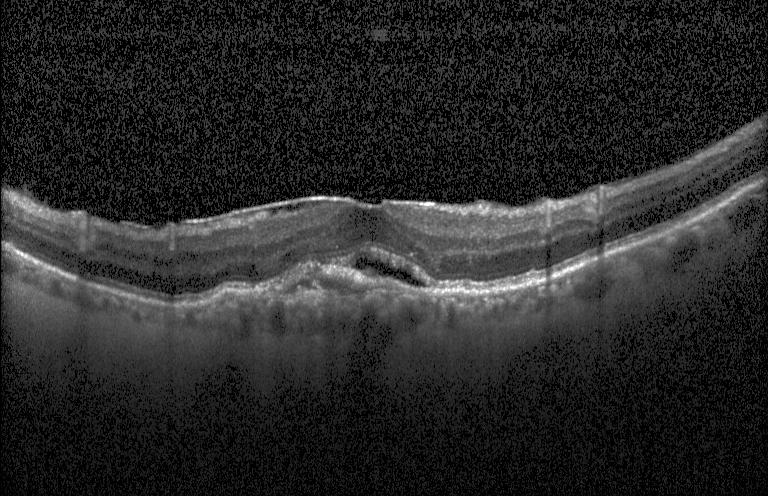 This B-scan demonstrates a choroidal neovascular membrane.